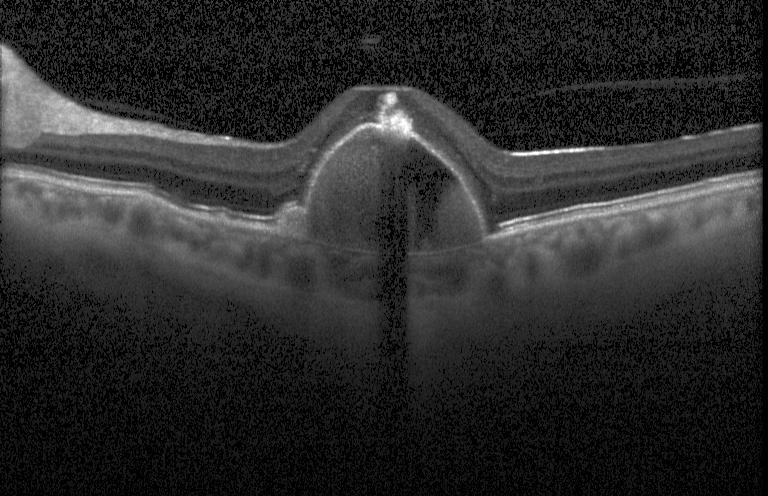

OCT line scan — Finding: a choroidal neovascular membrane.